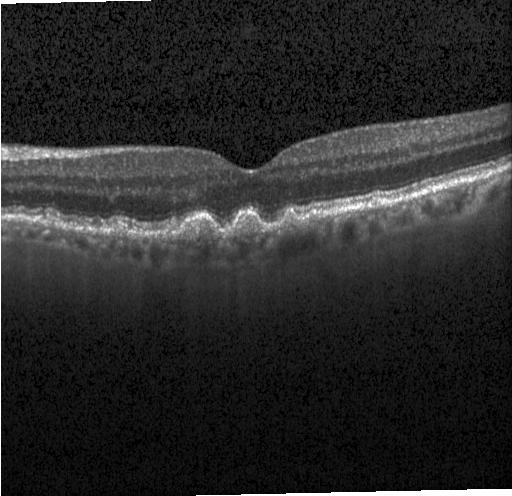

Assessment: multiple drusen.